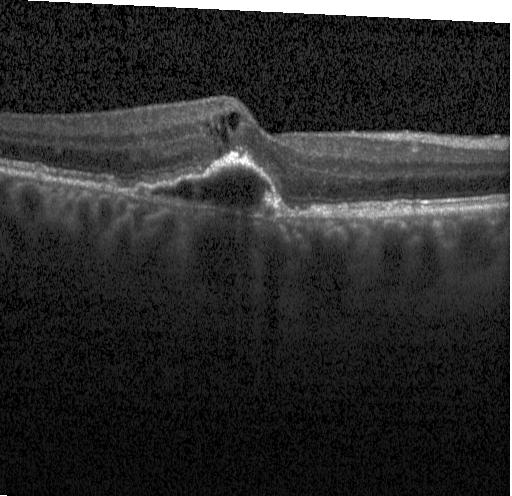

Acquired on a Heidelberg Spectralis, optical coherence tomography B-scan, spectral-domain OCT, fovea-centered. The scan shows choroidal neovascularization.